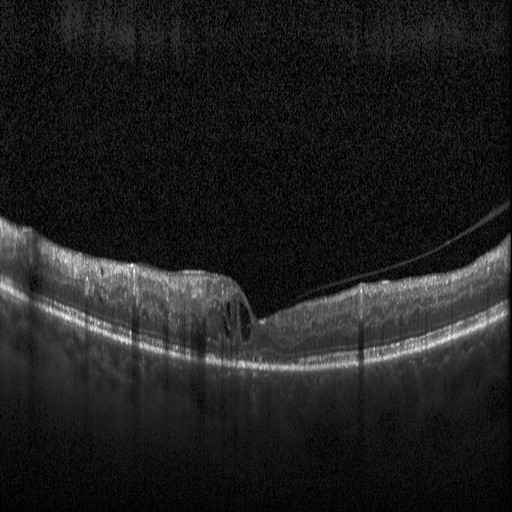 Heidelberg Spectralis OCT system · retinal OCT cross-section.
Impression: diabetic macular edema.